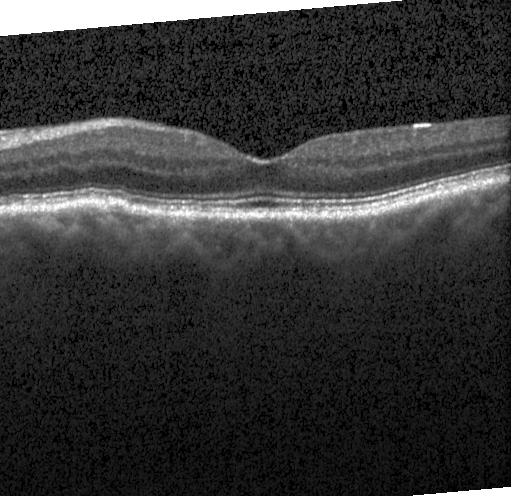

Centered on the fovea; optical coherence tomography scan — Impression: drusen.